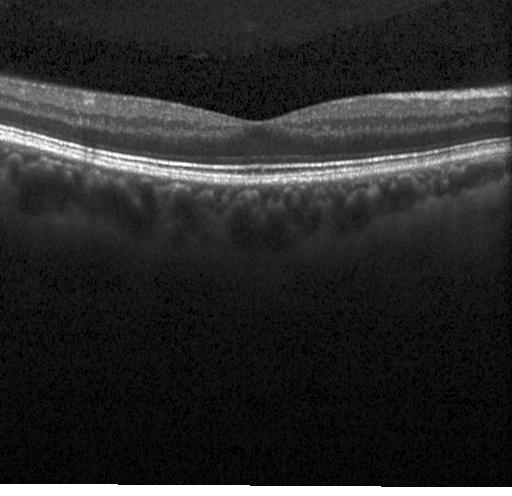

Retinal OCT cross-section. This B-scan demonstrates no choroidal neovascularization, no diabetic macular edema, and no drusen.